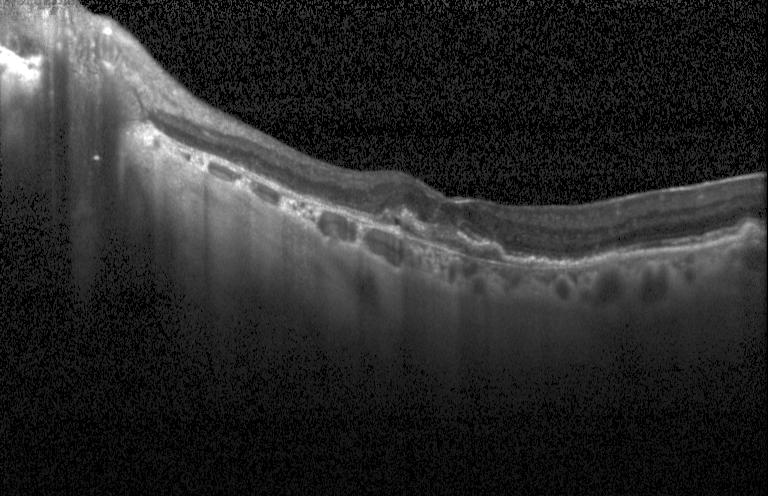

Heidelberg Spectralis OCT system · optical coherence tomography B-scan · spectral-domain OCT · fovea-centered.
The scan shows choroidal neovascularization (CNV).